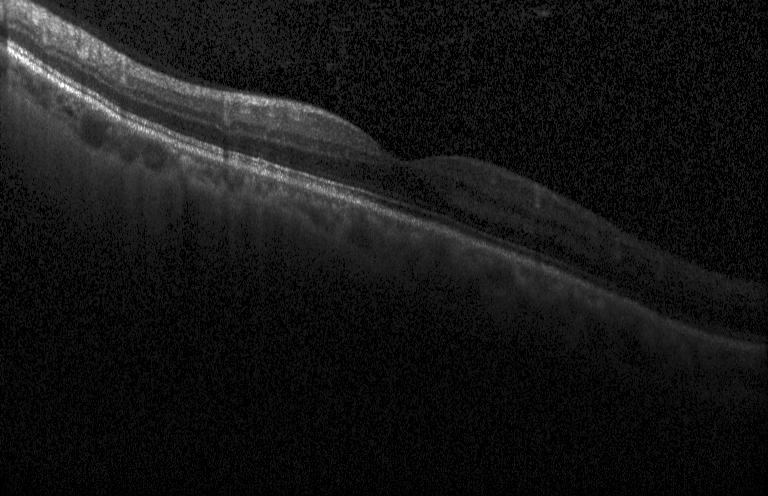
SD-OCT. Fovea-centered. Heidelberg Spectralis OCT system. Retinal OCT cross-section — OCT finding: neither CNV, DME, nor drusen.